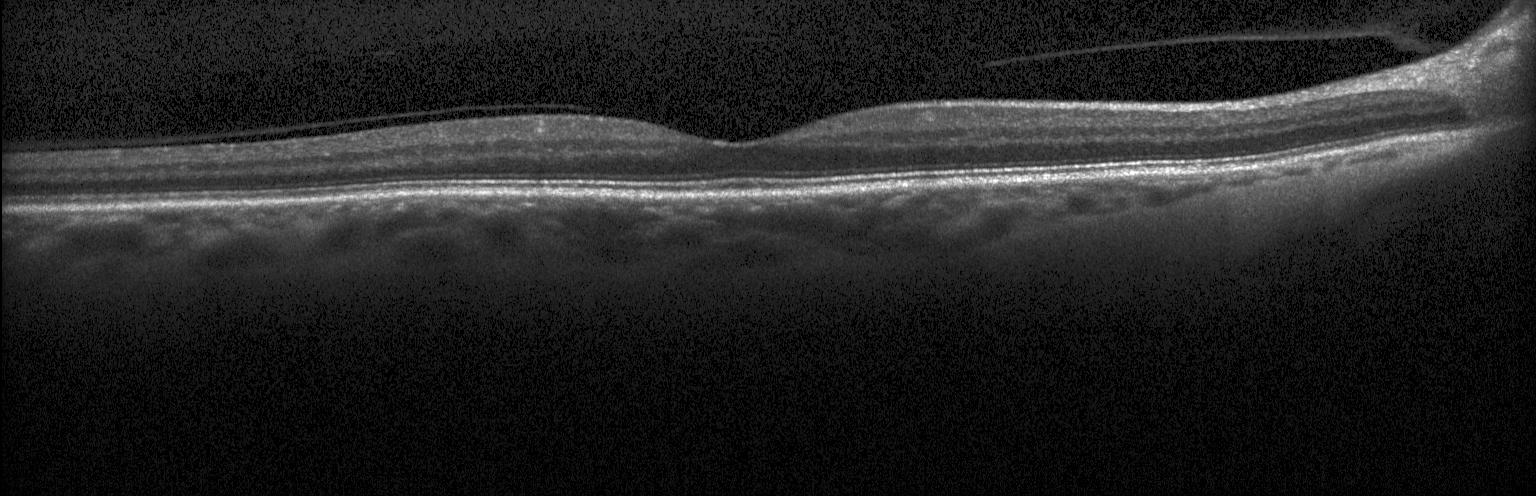

Spectral-domain optical coherence tomography · fovea-centered · retinal OCT B-scan — Finding: neither choroidal neovascularization, diabetic macular edema, nor drusen.